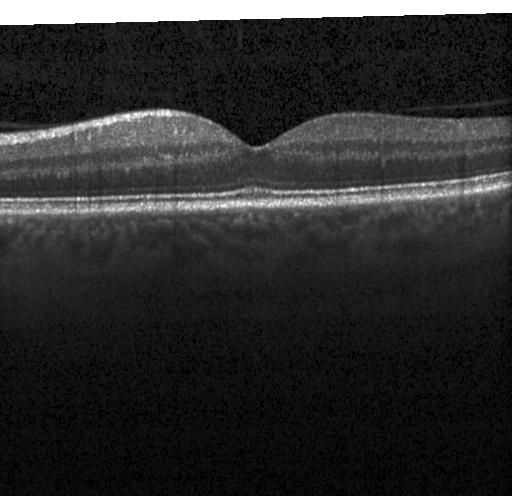 Assessment: no choroidal neovascularization, diabetic macular edema, or drusen.